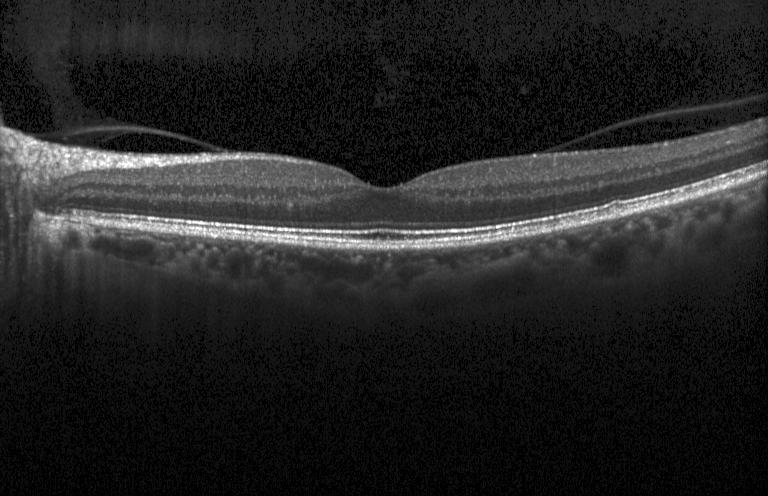
Fovea-centered; spectral-domain OCT; retinal OCT cross-section; instrument: Heidelberg Spectralis
OCT finding: no choroidal neovascularization, diabetic macular edema, or drusen.